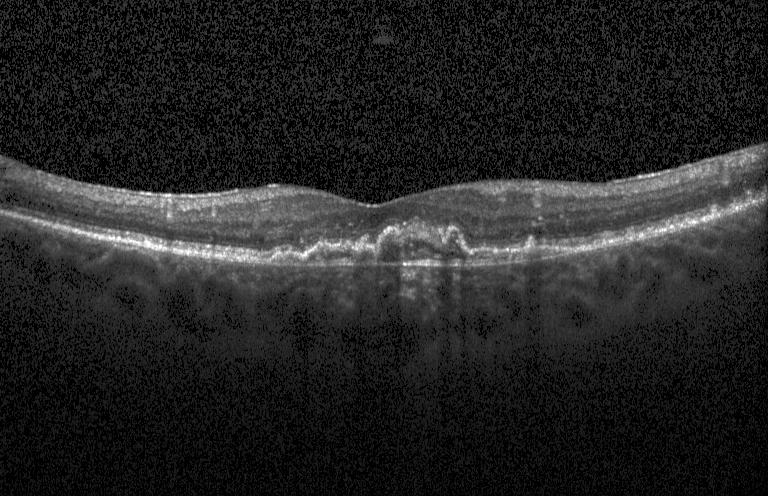
Optical coherence tomography B-scan — Assessment: a choroidal neovascular membrane.